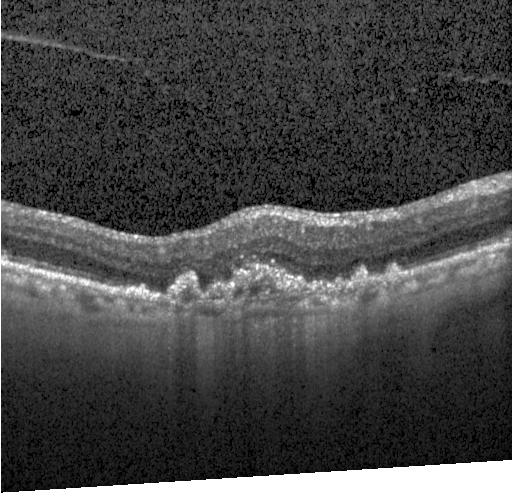
Assessment: CNV.